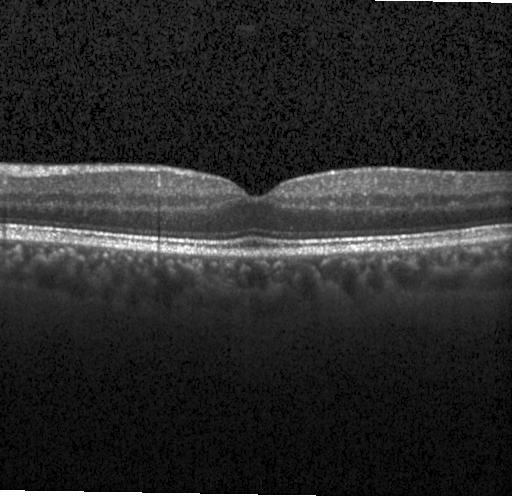 Instrument: Heidelberg Spectralis; OCT line scan; centered on the fovea. Assessment: no choroidal neovascularization, no diabetic macular edema, and no drusen.